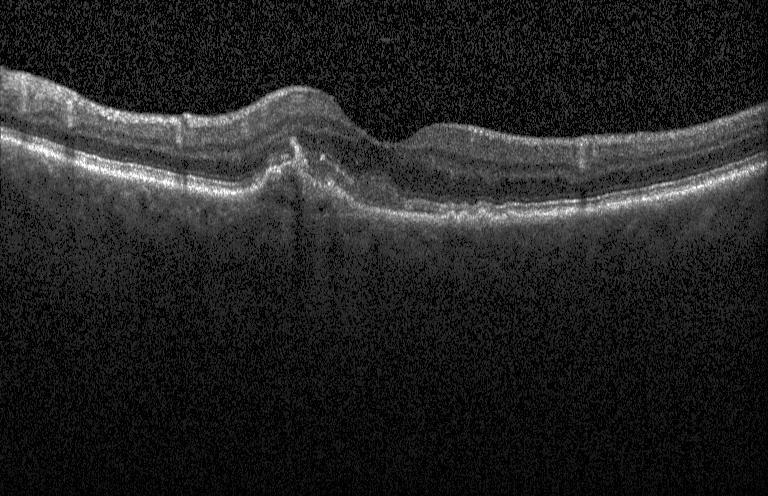

Macular OCT: choroidal neovascularization.